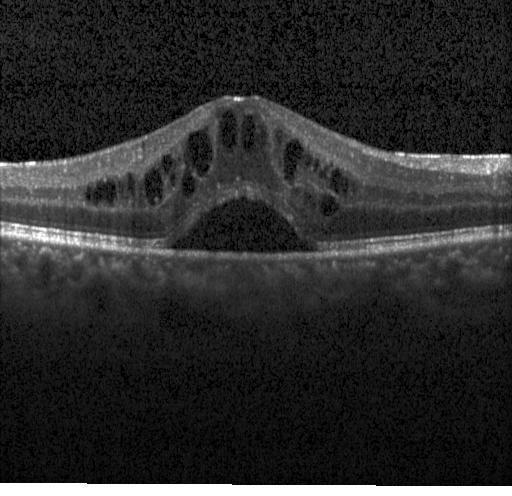 OCT B-scan showing diabetic macular edema (DME).